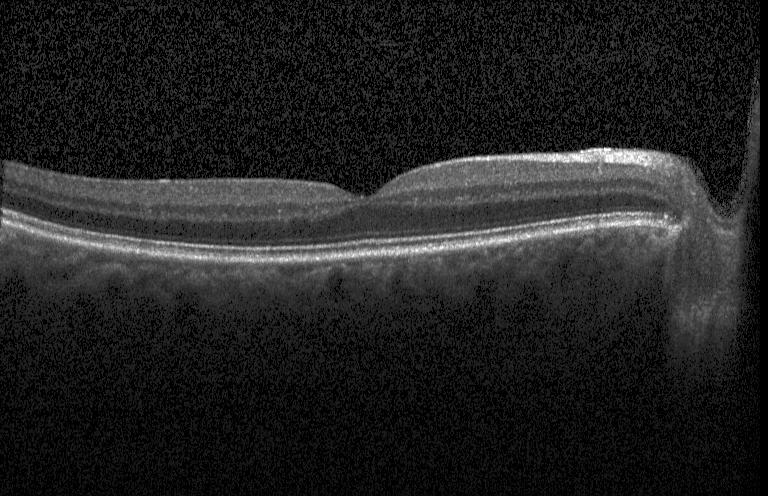

Fovea-centered; retinal OCT B-scan; Heidelberg Spectralis OCT system; spectral-domain optical coherence tomography. Diagnosis: no evidence of CNV, DME, or drusen.